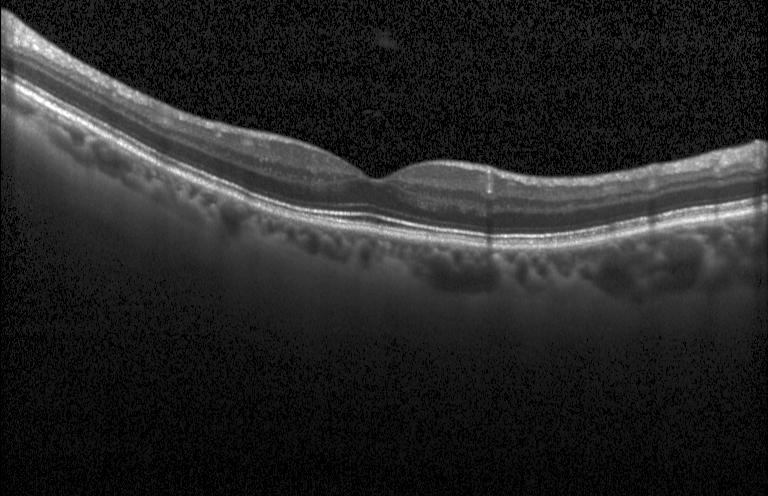 Impression: no choroidal neovascularization, diabetic macular edema, or drusen.